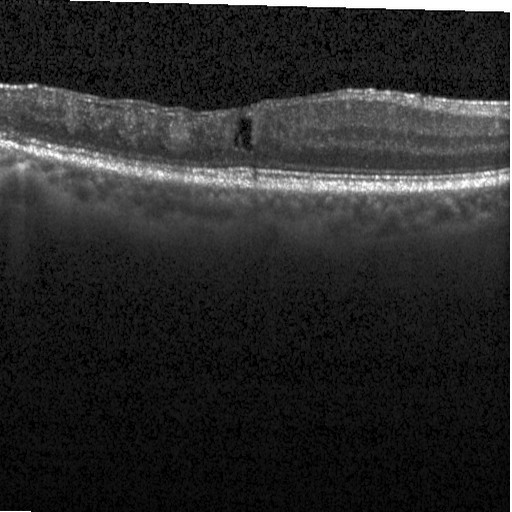 Horizontal scan through the fovea; SD-OCT; optical coherence tomography scan; acquired on a Heidelberg Spectralis. Assessment: DME.